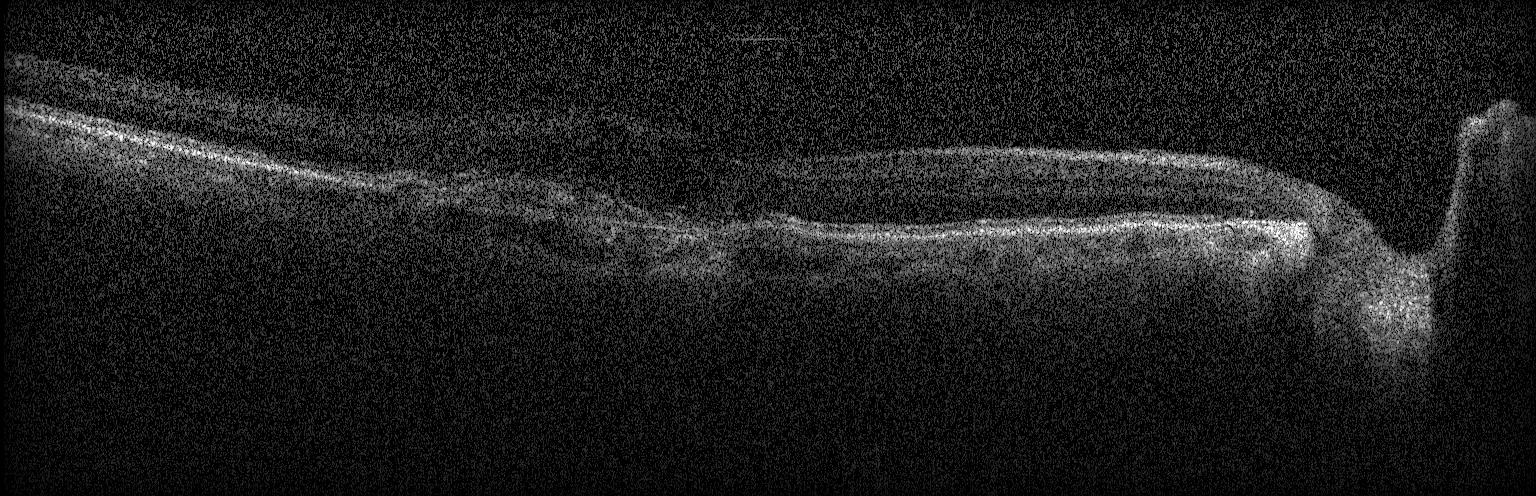
Retinal OCT cross-section
Dx: a choroidal neovascular membrane.